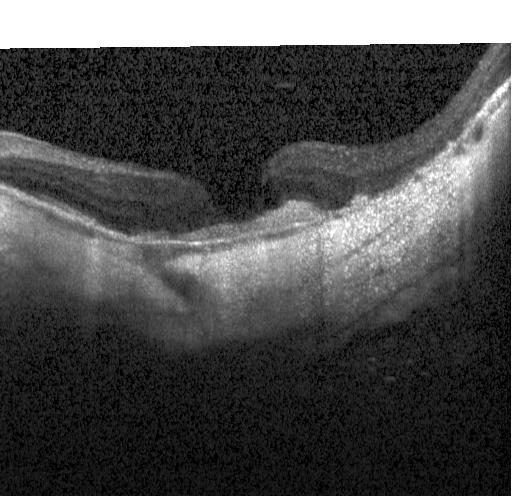
Heidelberg Spectralis. Retinal OCT cross-section. Macular scan. Spectral-domain optical coherence tomography — Finding: choroidal neovascularization (CNV).